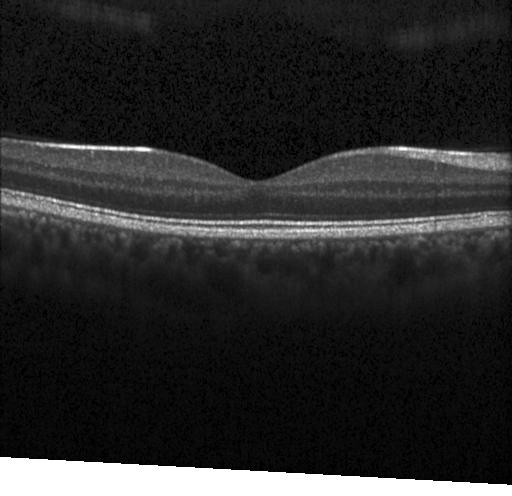 Finding: no choroidal neovascularization, no diabetic macular edema, and no drusen.